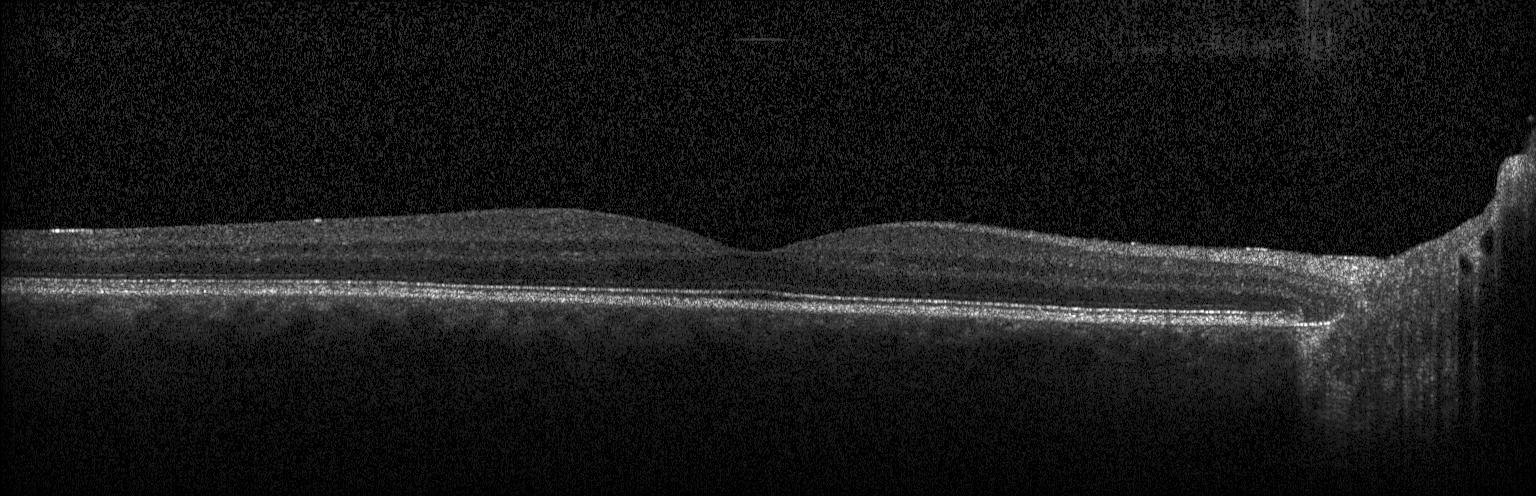 Retinal OCT B-scan; macular scan; spectral-domain optical coherence tomography; instrument: Heidelberg Spectralis.
Dx: neither choroidal neovascularization, diabetic macular edema, nor drusen.